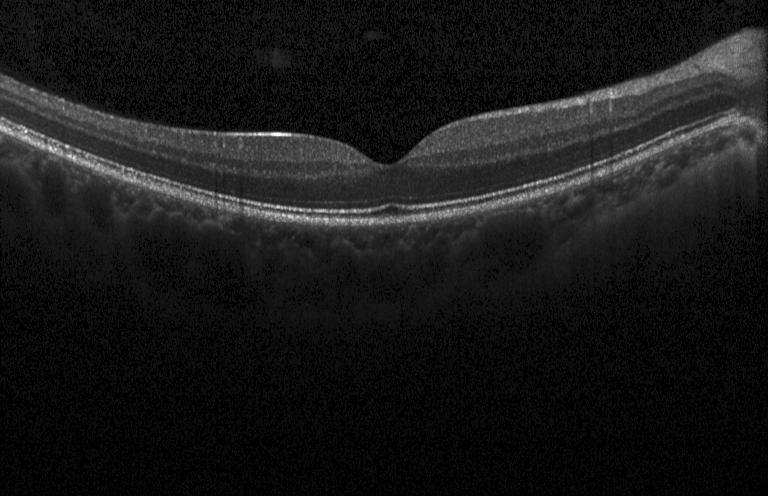

Spectral-domain OCT, retinal OCT cross-section, centered on the fovea
OCT finding: neither choroidal neovascularization, diabetic macular edema, nor drusen.